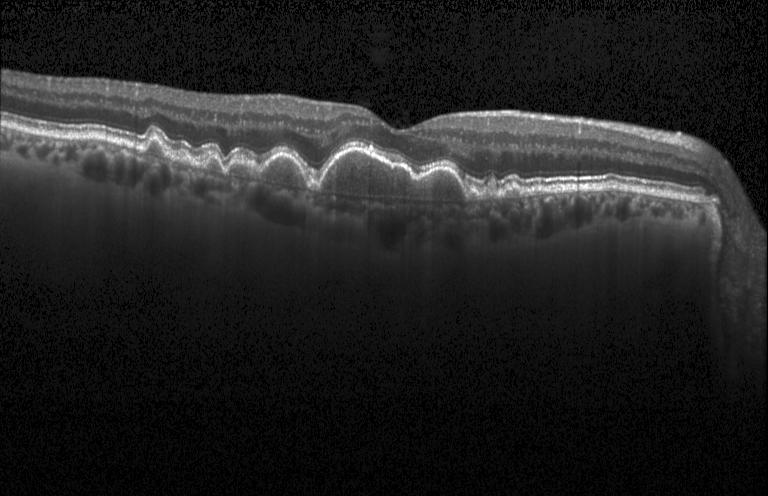

Heidelberg Spectralis OCT system. Horizontal scan through the fovea. Optical coherence tomography scan. SD-OCT — Assessment: sub-RPE drusenoid deposits.